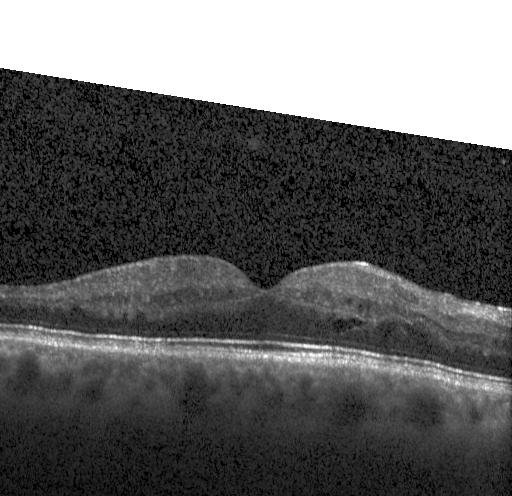 Impression: DME.